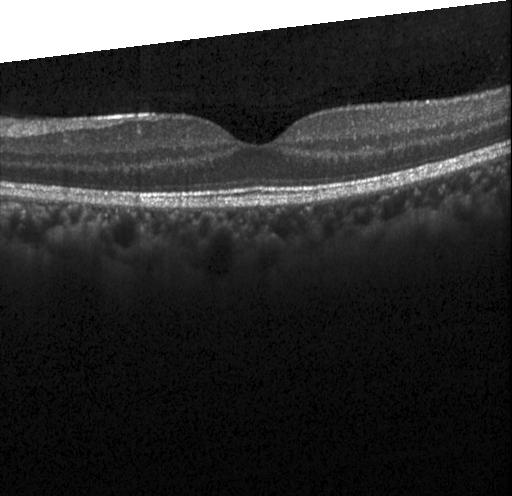

SD-OCT; macular scan; Heidelberg Spectralis OCT system; retinal OCT cross-section.
OCT finding: no choroidal neovascularization, no diabetic macular edema, and no drusen.